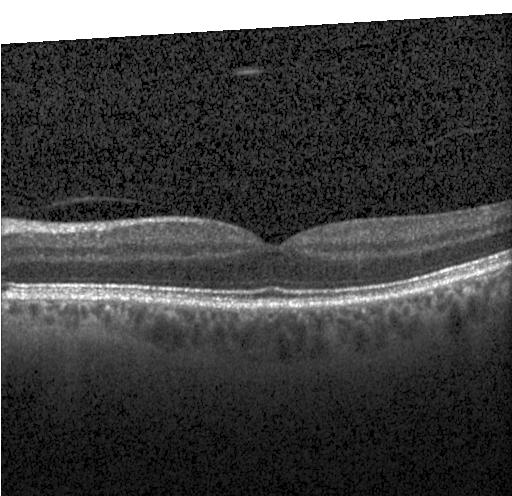
OCT finding: neither choroidal neovascularization, diabetic macular edema, nor drusen.